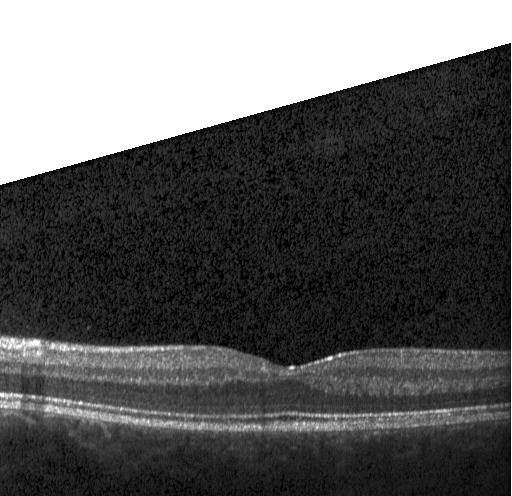
Retinal OCT cross-section showing no CNV, DME, or drusen.